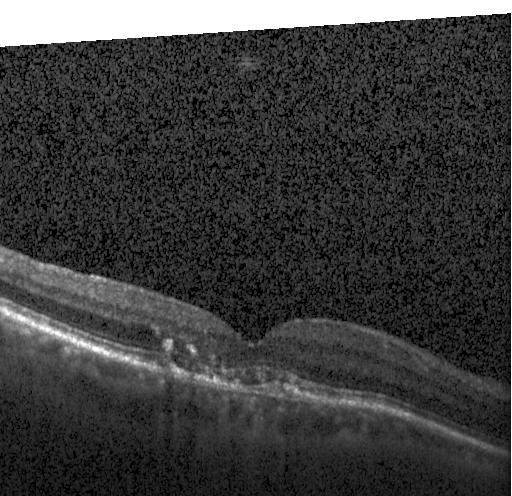
Acquired on a Heidelberg Spectralis · spectral-domain optical coherence tomography · optical coherence tomography B-scan · centered on the fovea. CNV.